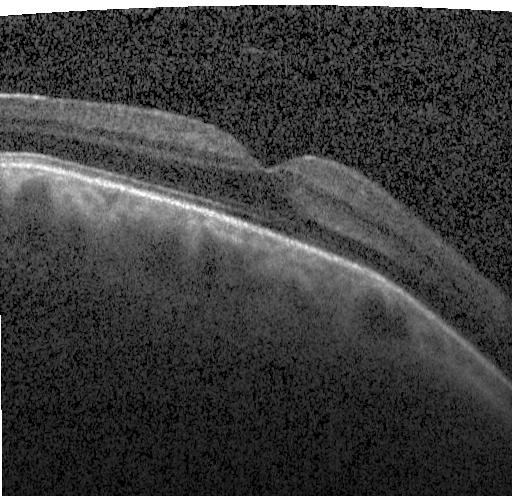 Retinal OCT cross-section. Diagnosis: no evidence of CNV, DME, or drusen.